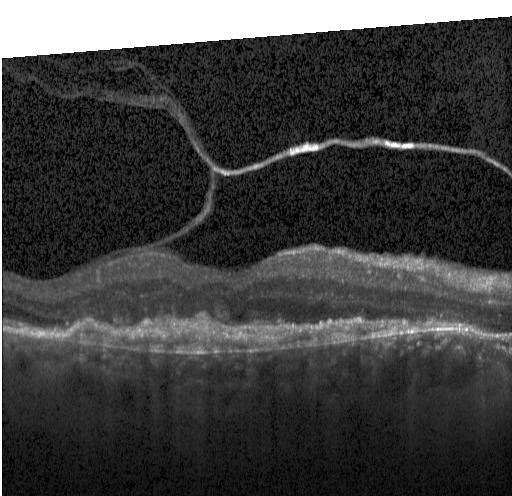 OCT line scan. Spectral-domain OCT. Choroidal neovascularization (CNV).